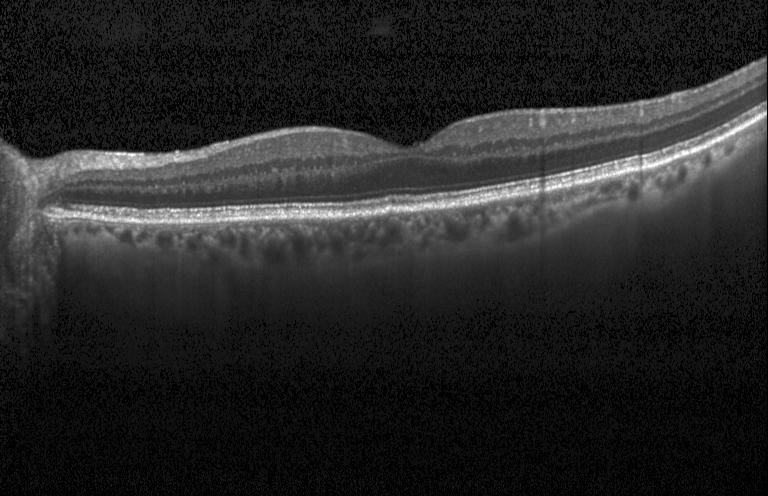
OCT line scan · instrument: Heidelberg Spectralis · centered on the fovea. Assessment: no evidence of choroidal neovascularization, diabetic macular edema, or drusen.